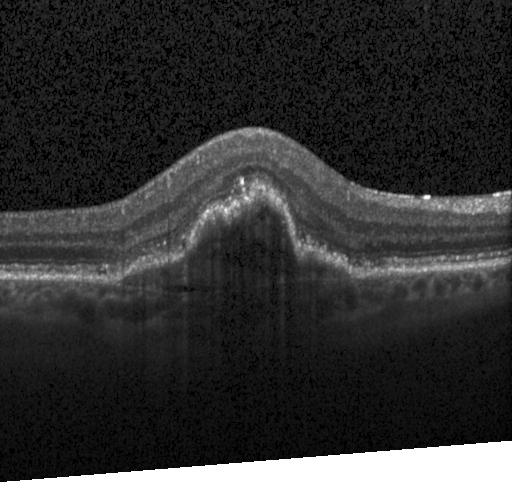

Finding: a choroidal neovascular membrane.